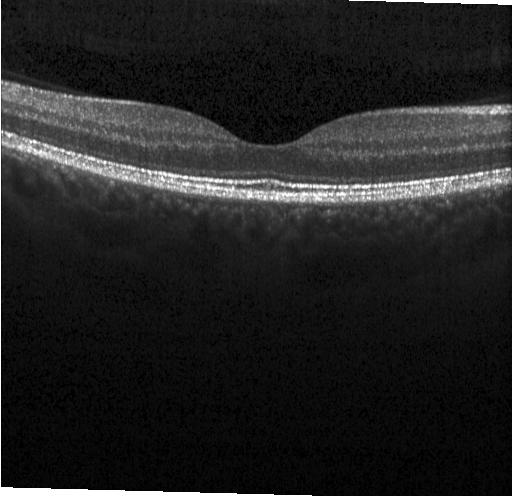
This B-scan demonstrates no choroidal neovascularization, no diabetic macular edema, and no drusen.